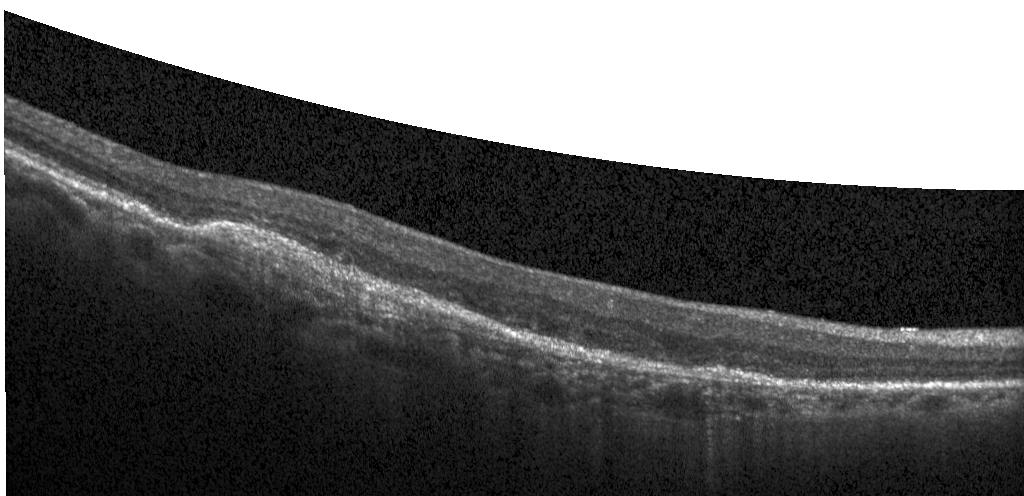 Instrument: Heidelberg Spectralis; centered on the fovea; retinal OCT cross-section — Dx: a choroidal neovascular membrane.